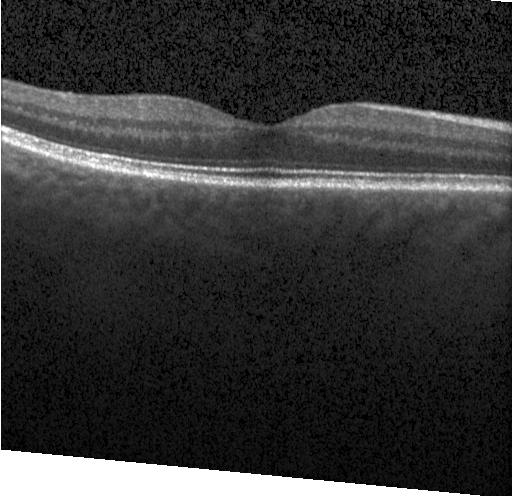
Optical coherence tomography B-scan, SD-OCT. Finding: no evidence of choroidal neovascularization, diabetic macular edema, or drusen.